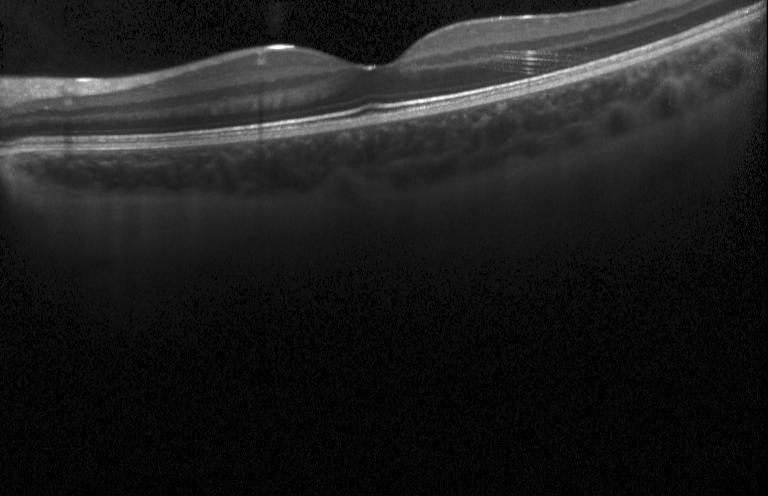
OCT finding: no evidence of choroidal neovascularization, diabetic macular edema, or drusen.